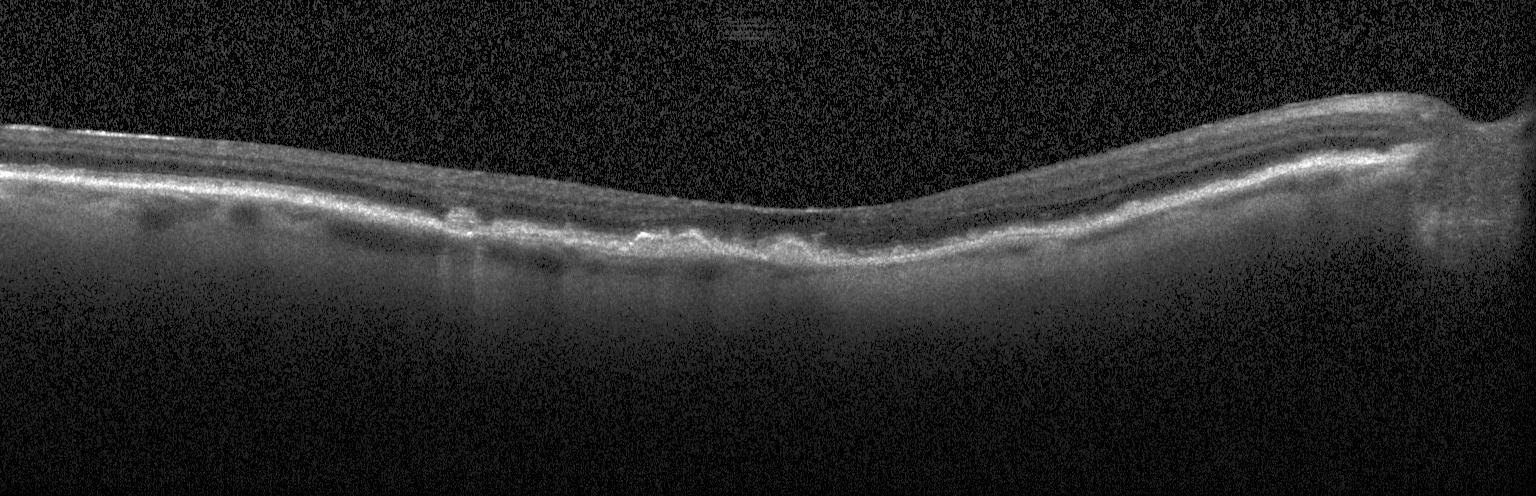

Retinal OCT B-scan
This B-scan demonstrates choroidal neovascularization (CNV).